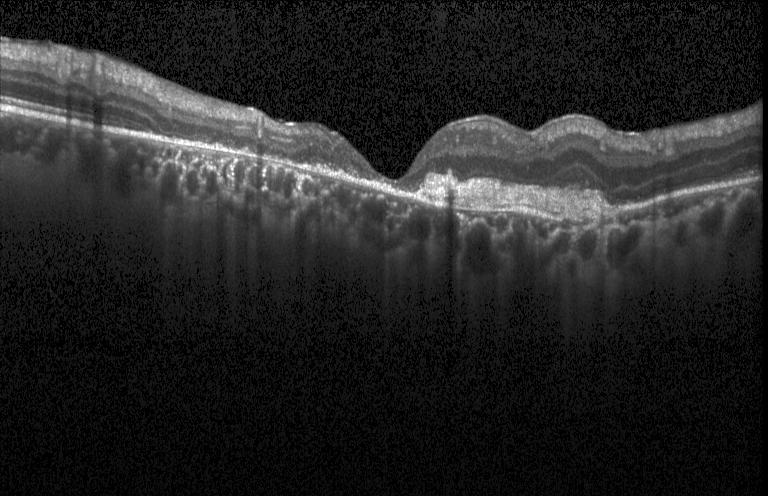 Instrument: Heidelberg Spectralis; SD-OCT; optical coherence tomography scan.
Finding: choroidal neovascularization.